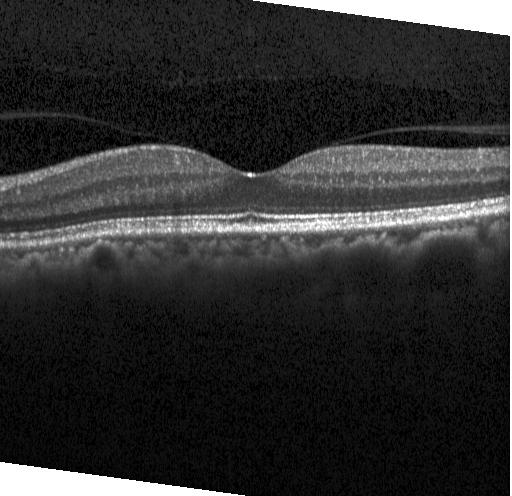 OCT scan showing no choroidal neovascularization, diabetic macular edema, or drusen.